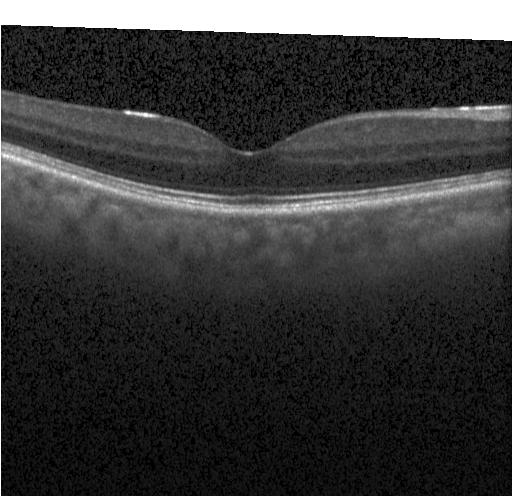

Centered on the fovea · retinal OCT B-scan · spectral-domain OCT · Heidelberg Spectralis — Assessment: no choroidal neovascularization, no diabetic macular edema, and no drusen.